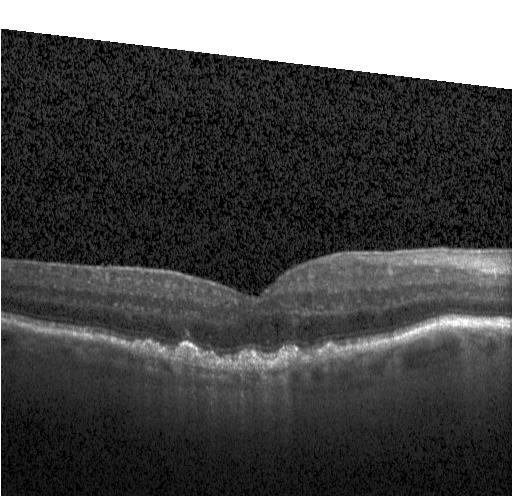

SD-OCT. Retinal OCT cross-section
Impression: a choroidal neovascular membrane.